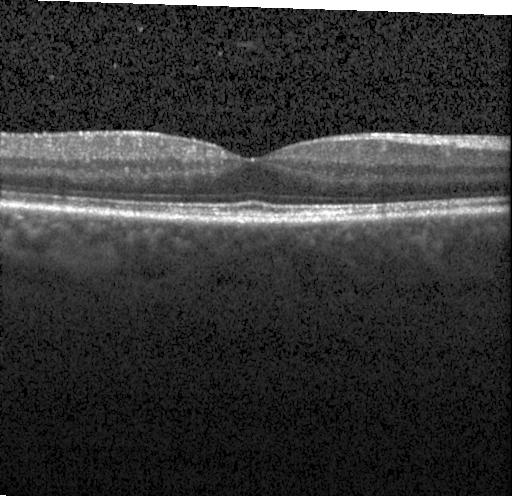
Spectral-domain OCT, optical coherence tomography B-scan — Dx: no choroidal neovascularization, diabetic macular edema, or drusen.